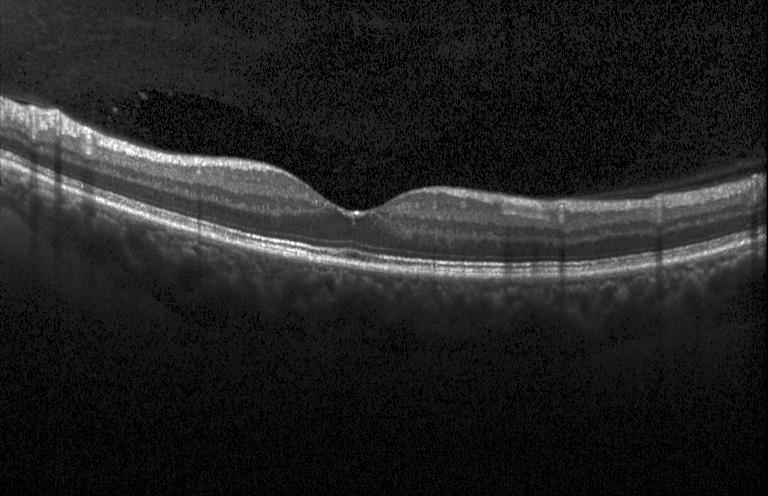 Fovea-centered, SD-OCT, instrument: Heidelberg Spectralis, OCT line scan — Diagnosis: no CNV, DME, or drusen.